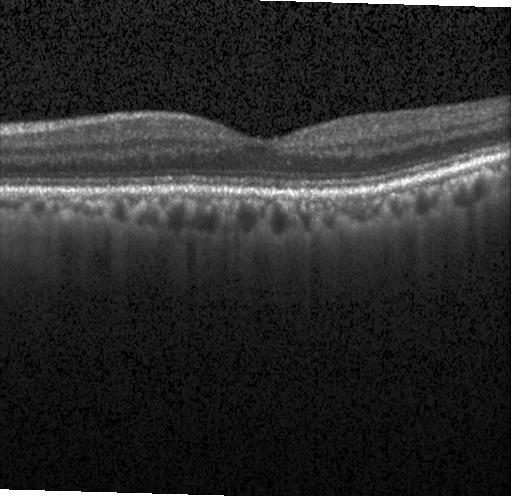
Heidelberg Spectralis OCT system. OCT line scan. Through the macula — Assessment: neither choroidal neovascularization, diabetic macular edema, nor drusen.